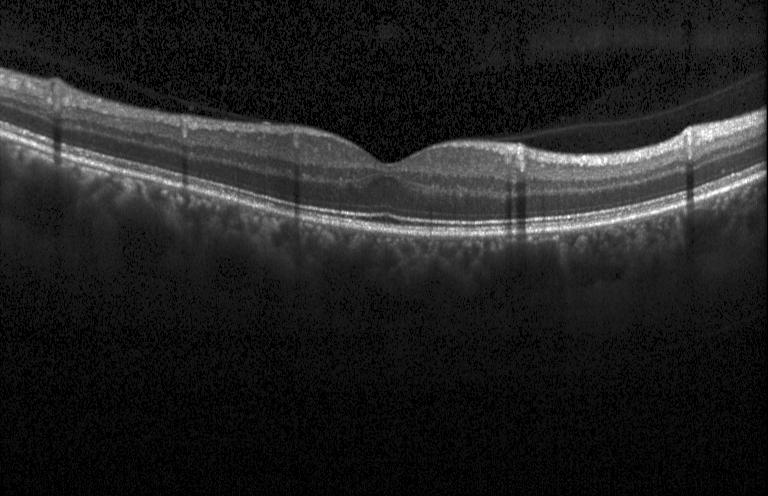
OCT line scan, Heidelberg Spectralis, spectral-domain OCT, through the macula — Diagnosis: no choroidal neovascularization, diabetic macular edema, or drusen.